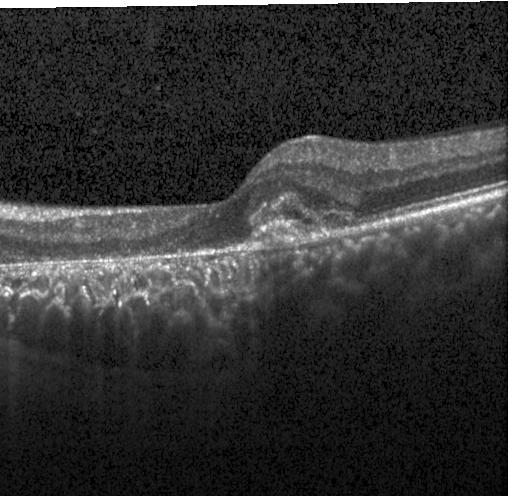 OCT finding: a choroidal neovascular membrane.